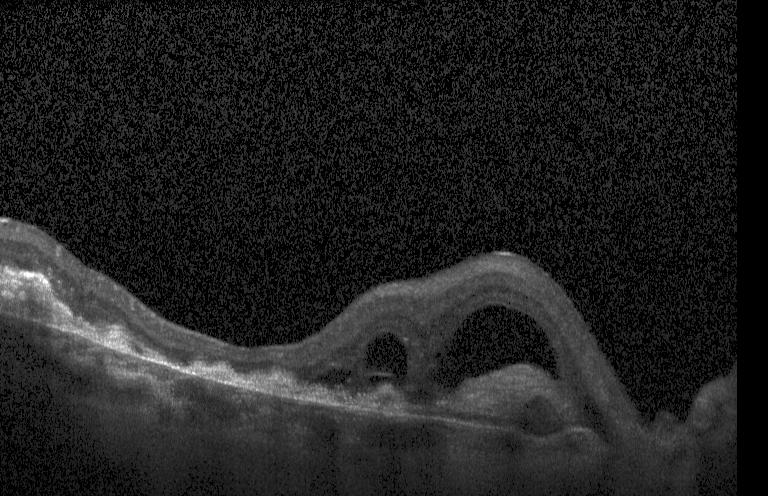

Fovea-centered · OCT line scan — OCT finding: a choroidal neovascular membrane.